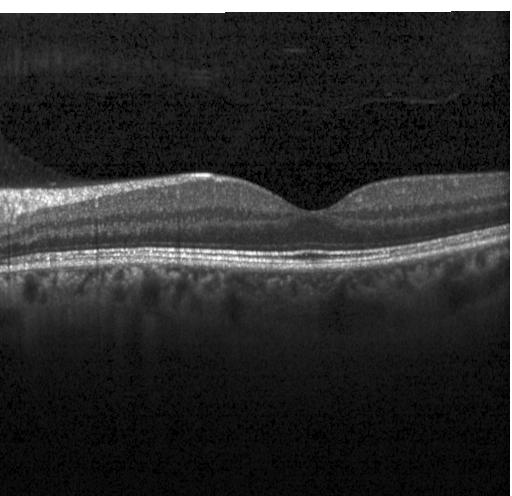
Spectral-domain optical coherence tomography · retinal OCT B-scan · centered on the fovea · Heidelberg Spectralis
Impression: neither choroidal neovascularization, diabetic macular edema, nor drusen.